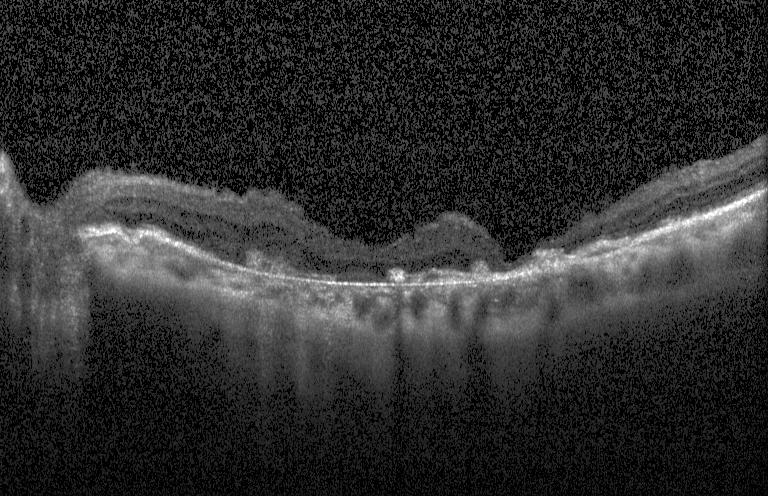
Retinal OCT B-scan, instrument: Heidelberg Spectralis, macular scan
Macular OCT: choroidal neovascularization.